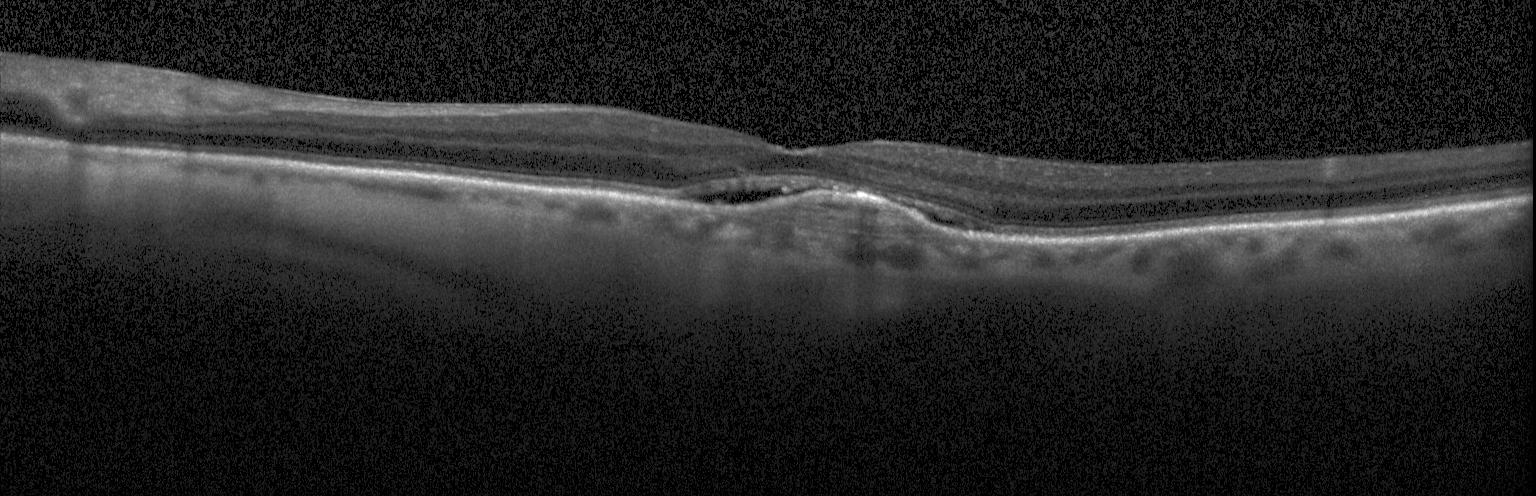

Finding: choroidal neovascularization (CNV).